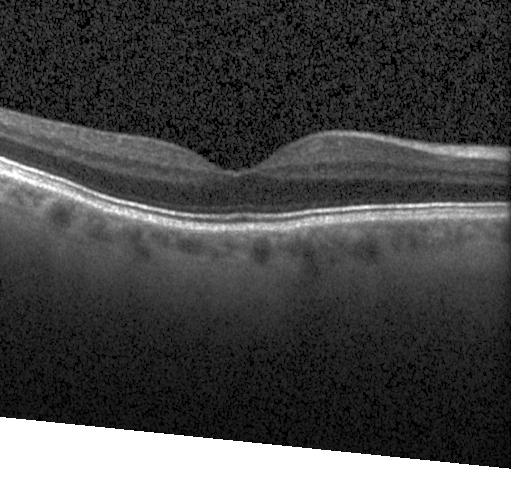

Optical coherence tomography scan · spectral-domain OCT · fovea-centered · Heidelberg Spectralis. Impression: no CNV, DME, or drusen.